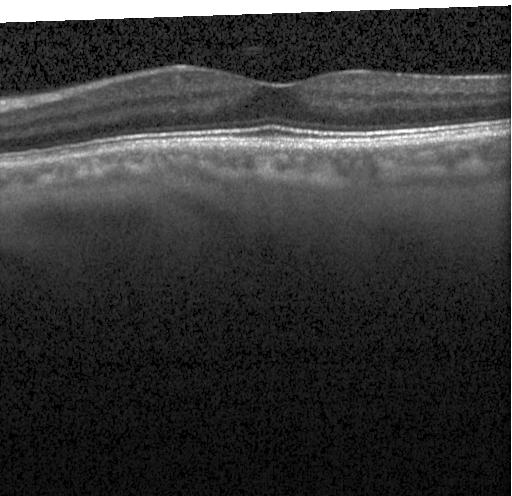 Retinal OCT B-scan, spectral-domain optical coherence tomography, Heidelberg Spectralis OCT system, centered on the fovea.
The scan shows no evidence of CNV, DME, or drusen.